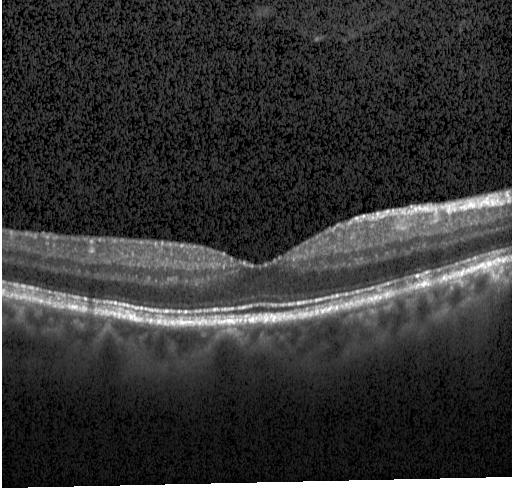
SD-OCT, optical coherence tomography scan, instrument: Heidelberg Spectralis
Assessment: no CNV, no DME, and no drusen.